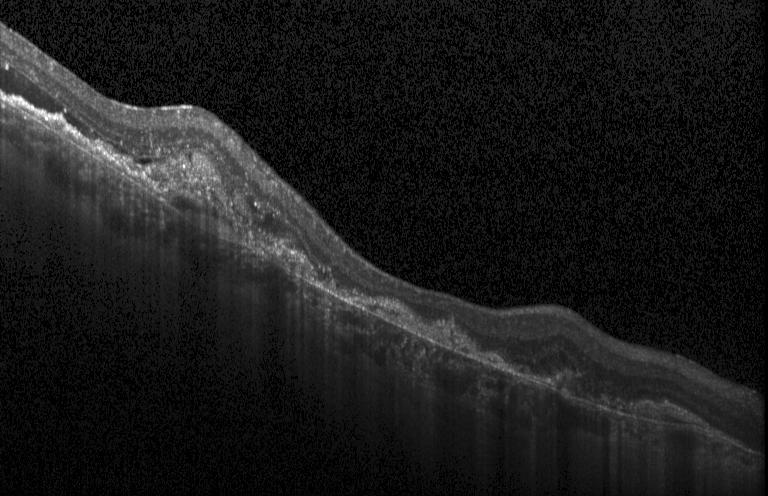
Horizontal scan through the fovea. Heidelberg Spectralis. OCT B-scan
Impression: a choroidal neovascular membrane.